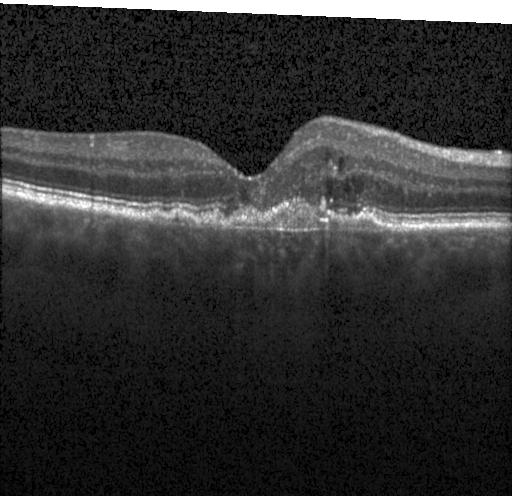
Optical coherence tomography scan; spectral-domain OCT
The scan shows a choroidal neovascular membrane.